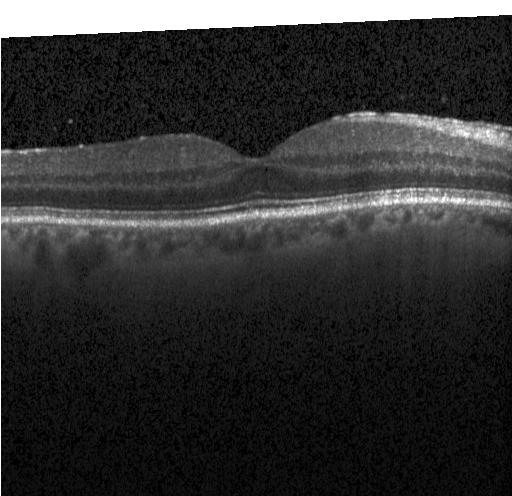
OCT scan showing neither choroidal neovascularization, diabetic macular edema, nor drusen.